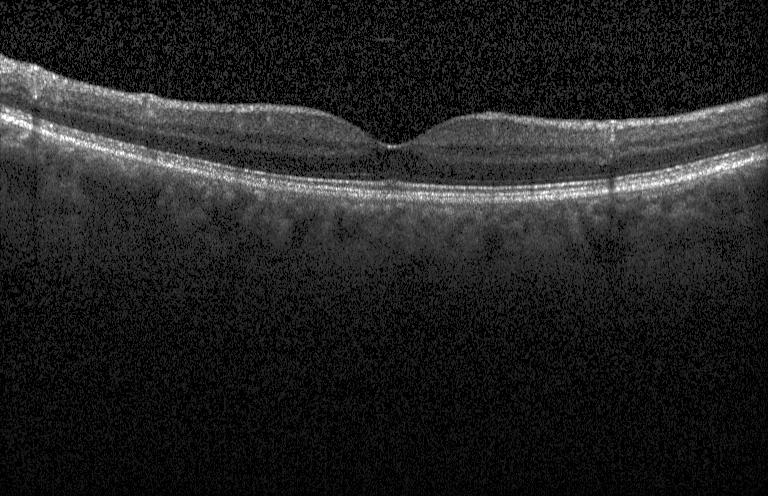

The scan shows neither choroidal neovascularization, diabetic macular edema, nor drusen.